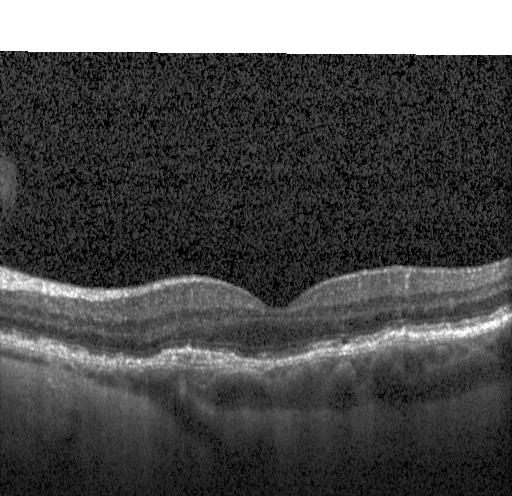
This B-scan demonstrates a choroidal neovascular membrane.